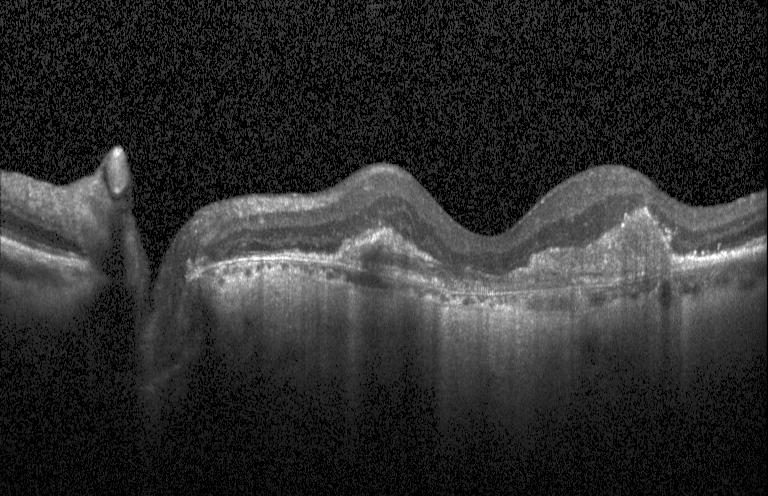
OCT scan showing a choroidal neovascular membrane.